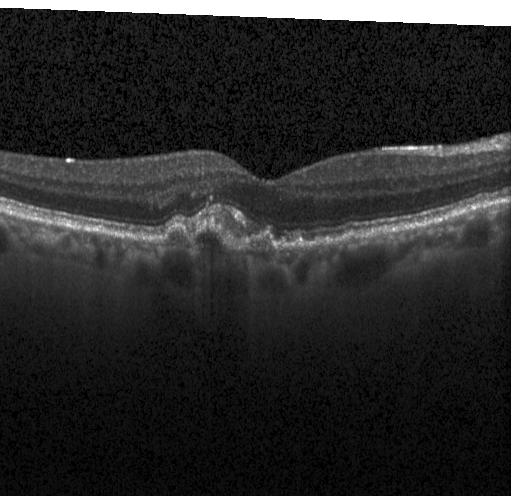 Impression: a choroidal neovascular membrane.